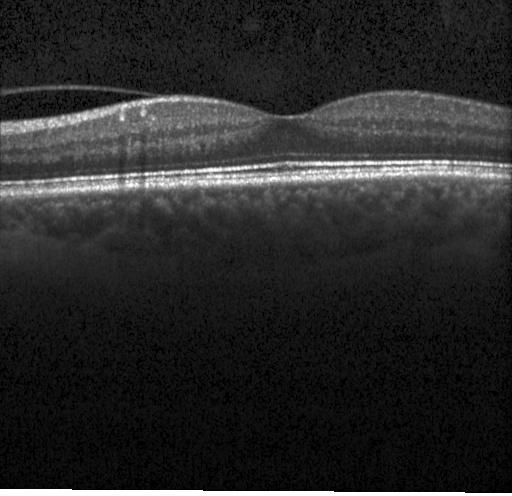

Instrument: Heidelberg Spectralis. Retinal OCT B-scan. Through the macula. Spectral-domain optical coherence tomography
OCT finding: no choroidal neovascularization, diabetic macular edema, or drusen.